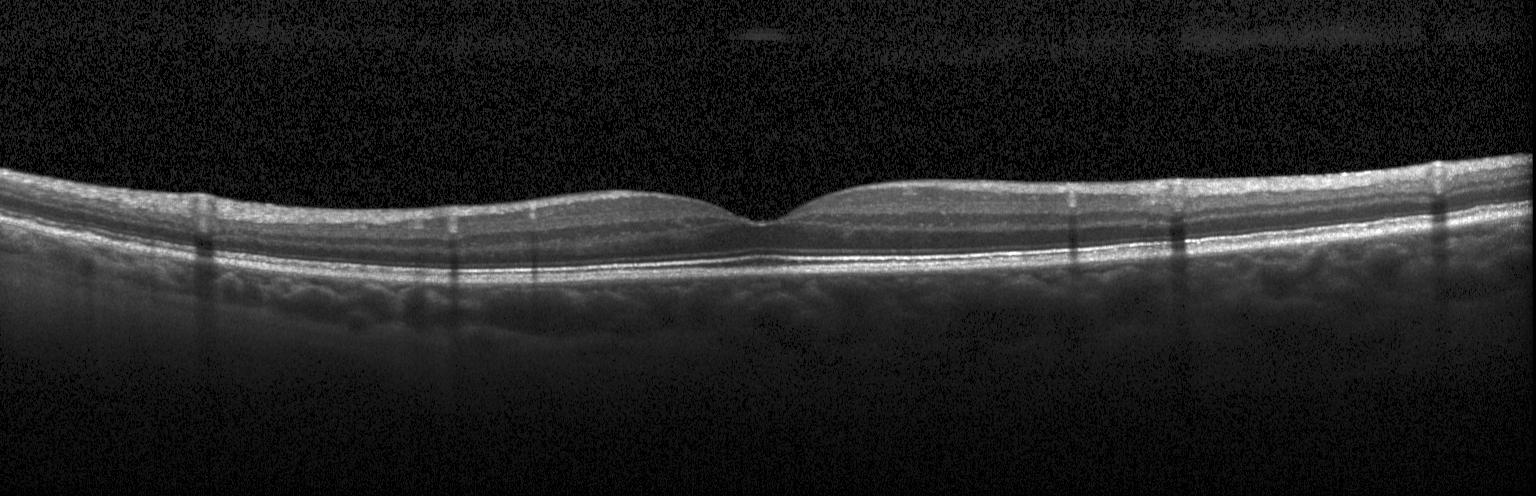 OCT scan showing no choroidal neovascularization, diabetic macular edema, or drusen.